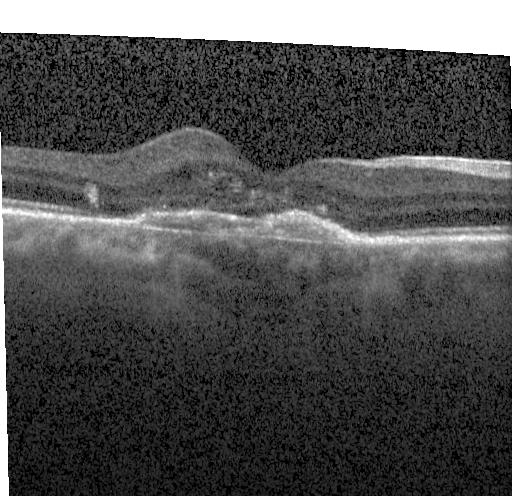 Retinal OCT cross-section showing a choroidal neovascular membrane.